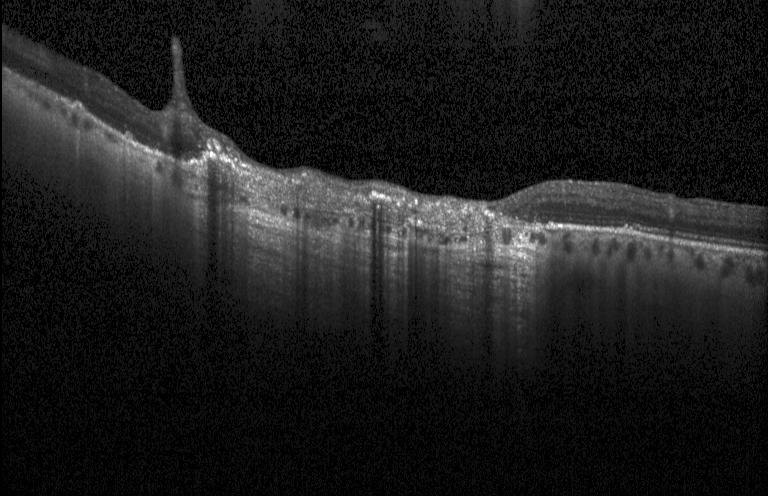 Impression: a choroidal neovascular membrane.